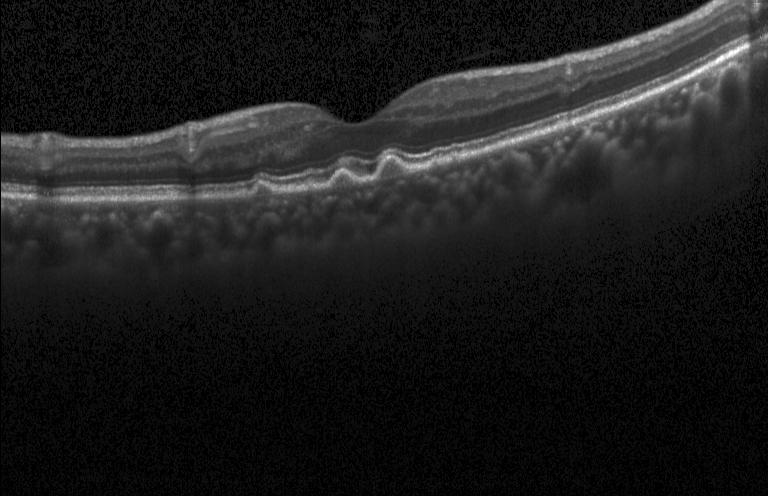
Assessment: multiple drusen.